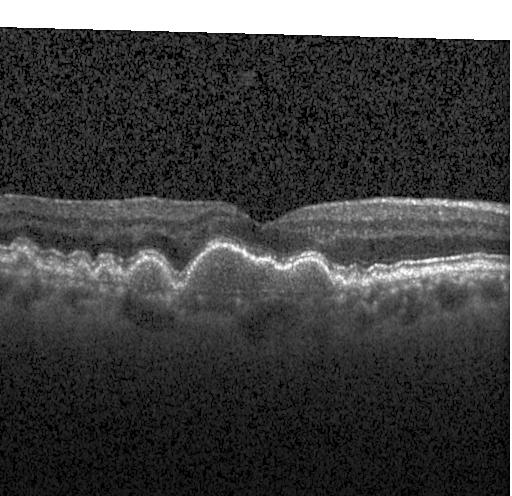
SD-OCT, optical coherence tomography scan, fovea-centered, Heidelberg Spectralis OCT system. Finding: multiple drusen.